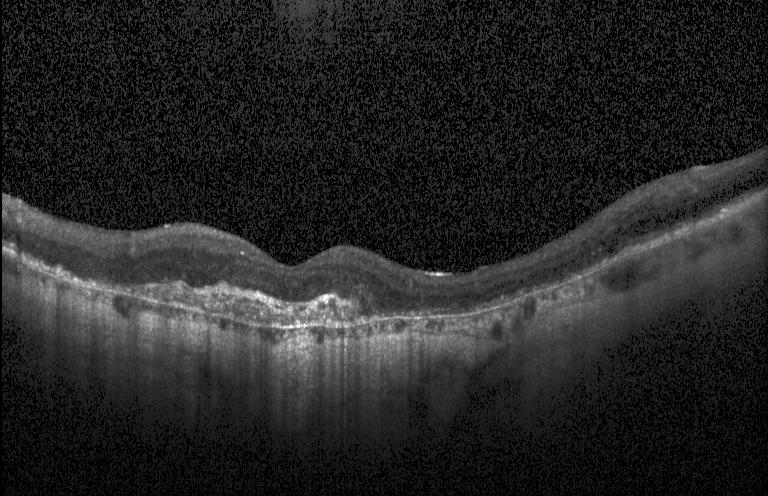 OCT scan showing a choroidal neovascular membrane.